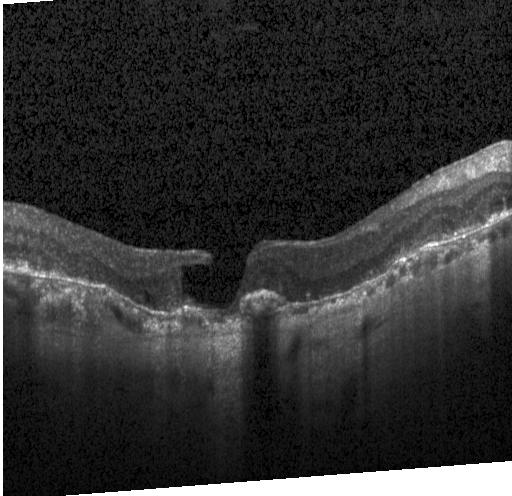
Macular OCT: a choroidal neovascular membrane.